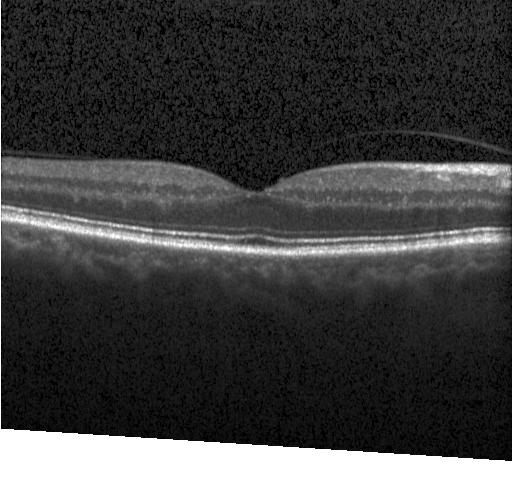 Assessment: no evidence of choroidal neovascularization, diabetic macular edema, or drusen.